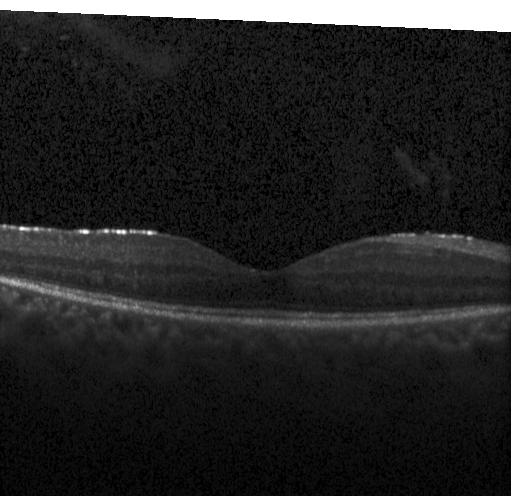
Instrument: Heidelberg Spectralis. Optical coherence tomography scan.
Assessment: neither choroidal neovascularization, diabetic macular edema, nor drusen.